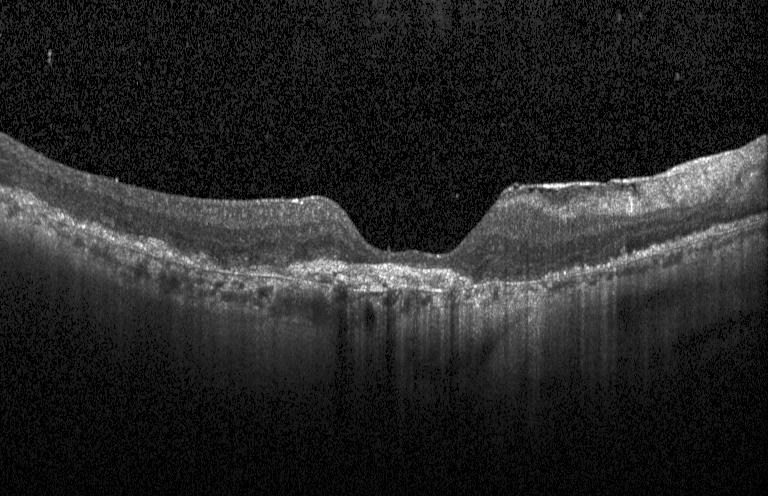

Optical coherence tomography B-scan, through the macula, spectral-domain OCT.
This B-scan demonstrates a choroidal neovascular membrane.